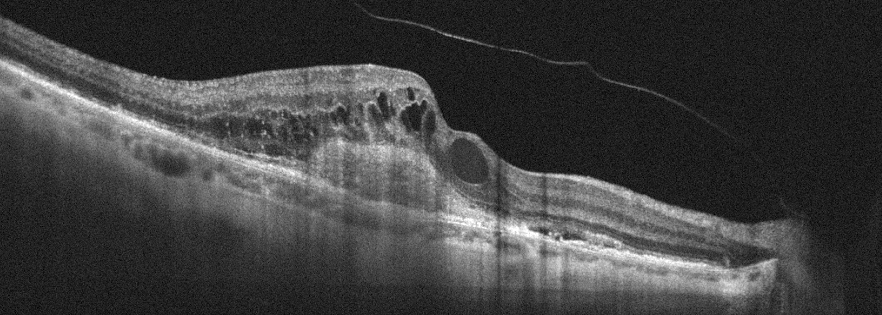 OCT B-scan; oculus dexter; fovea-centered. Diagnosis: AMD.